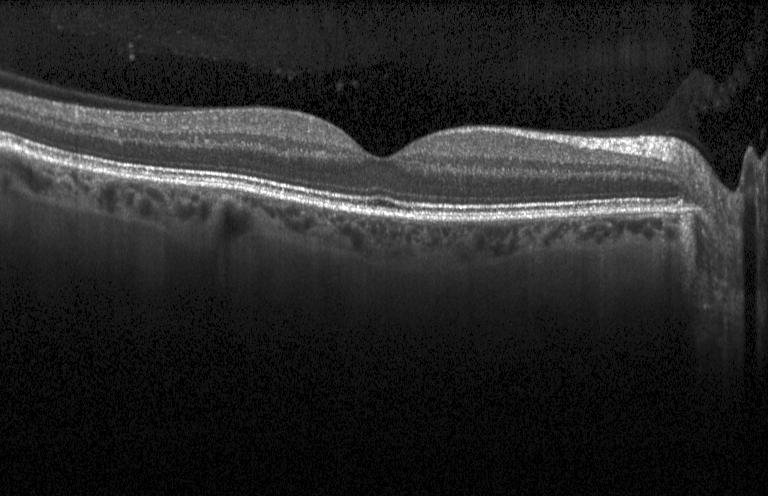
Heidelberg Spectralis. Spectral-domain OCT. OCT line scan. Fovea-centered.
No CNV, no DME, and no drusen.